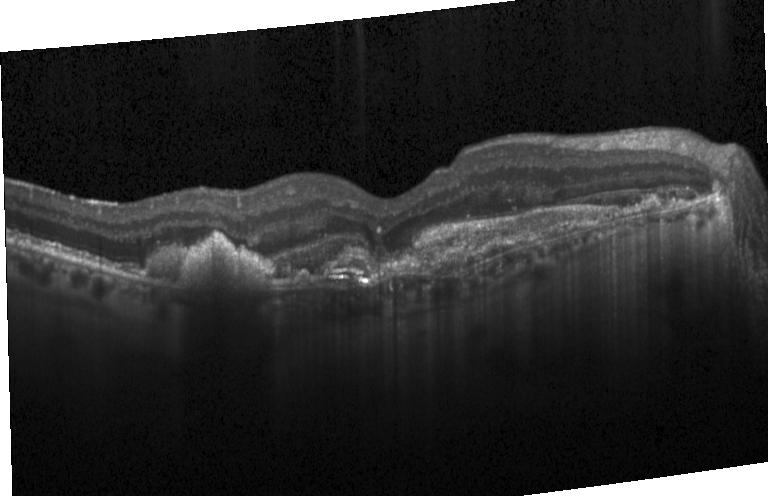 Optical coherence tomography B-scan · instrument: Heidelberg Spectralis · spectral-domain OCT.
Impression: a choroidal neovascular membrane.